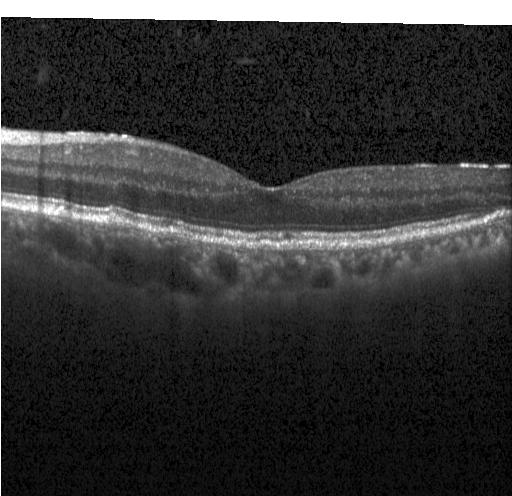 OCT B-scan; horizontal scan through the fovea — Assessment: sub-RPE drusenoid deposits.